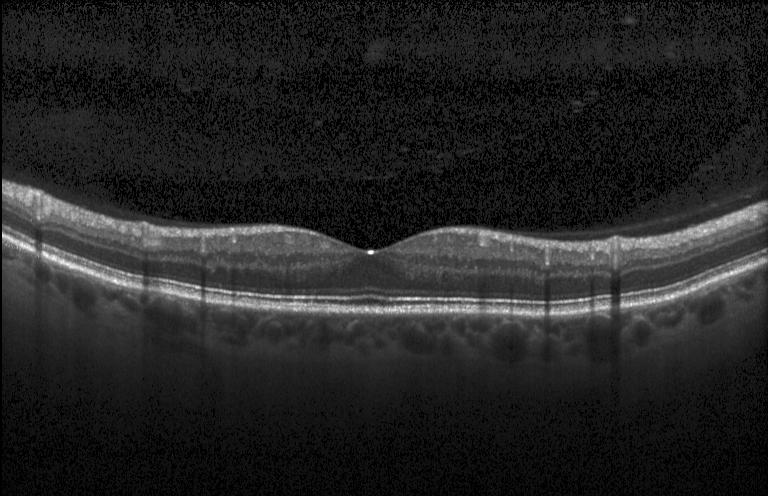

Optical coherence tomography B-scan · SD-OCT — Finding: no CNV, DME, or drusen.